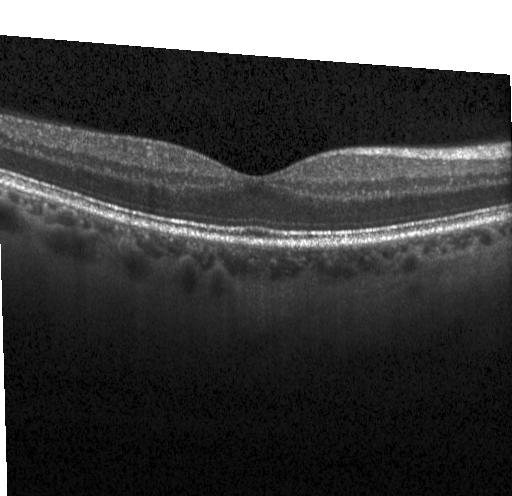

OCT B-scan; centered on the fovea; instrument: Heidelberg Spectralis.
Impression: no choroidal neovascularization, no diabetic macular edema, and no drusen.